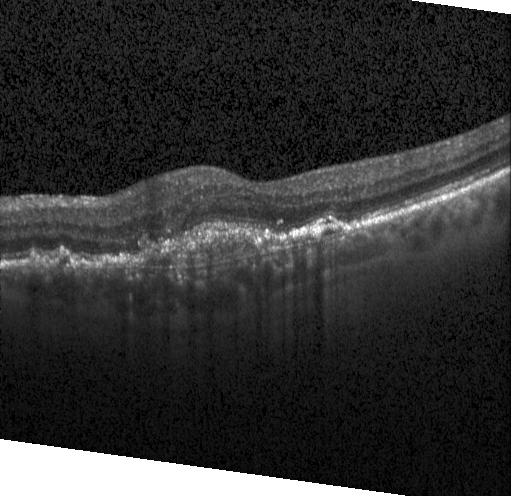

Fovea-centered · SD-OCT · OCT B-scan. This B-scan demonstrates choroidal neovascularization.